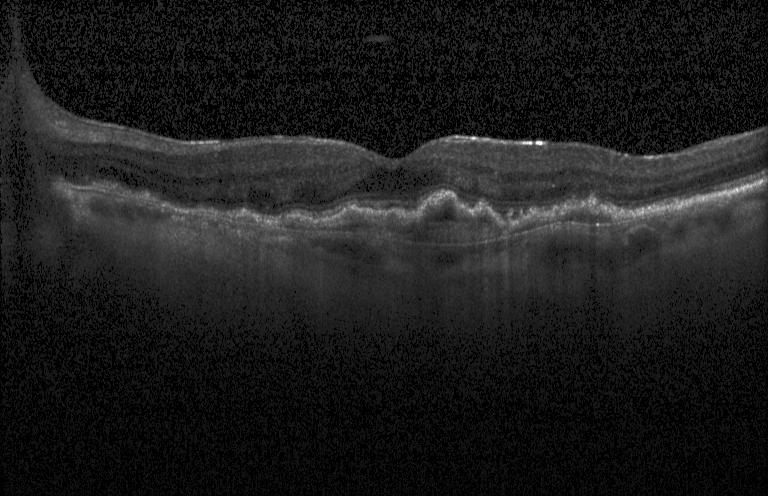

Retinal OCT cross-section
Diagnosis: a choroidal neovascular membrane.